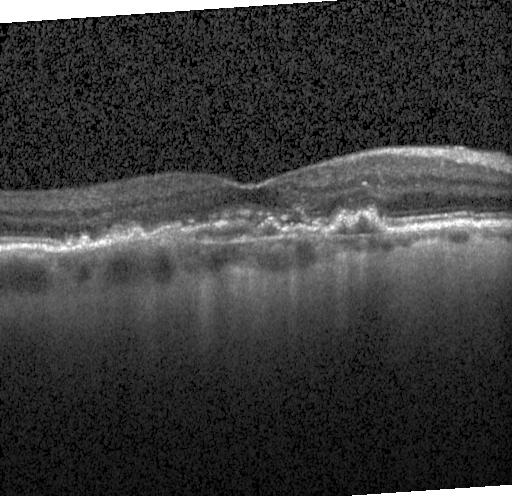
Diagnosis: a choroidal neovascular membrane.